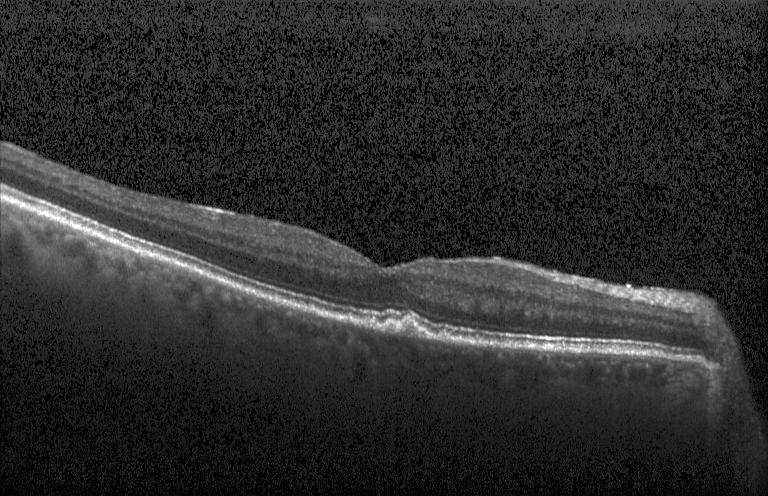
OCT B-scan. OCT finding: sub-RPE drusenoid deposits.